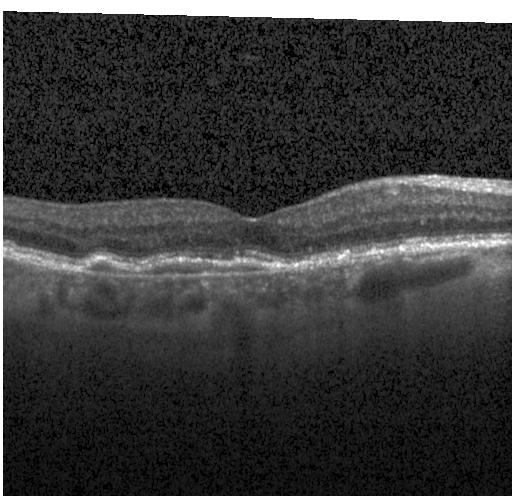
Retinal OCT cross-section showing choroidal neovascularization.